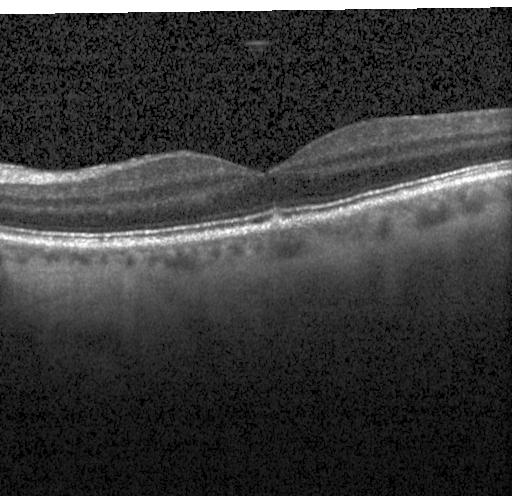 Horizontal scan through the fovea. Heidelberg Spectralis. Retinal OCT cross-section. Spectral-domain optical coherence tomography.
Macular OCT: multiple drusen.